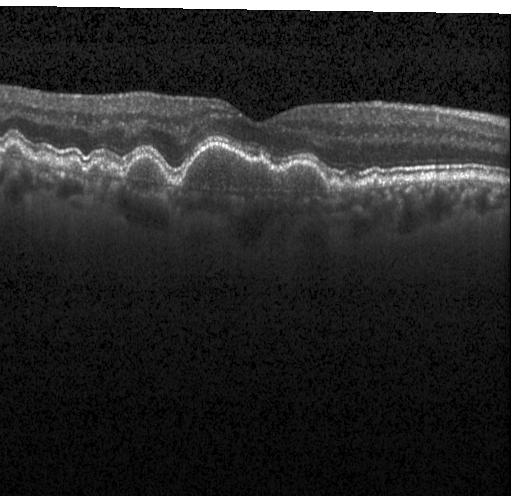

Retinal OCT B-scan · fovea-centered. Impression: multiple drusen.